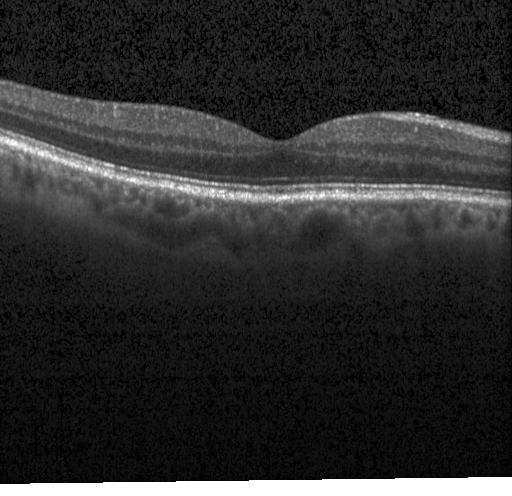 Macular scan. Retinal OCT B-scan. Spectral-domain OCT. This B-scan demonstrates neither choroidal neovascularization, diabetic macular edema, nor drusen.